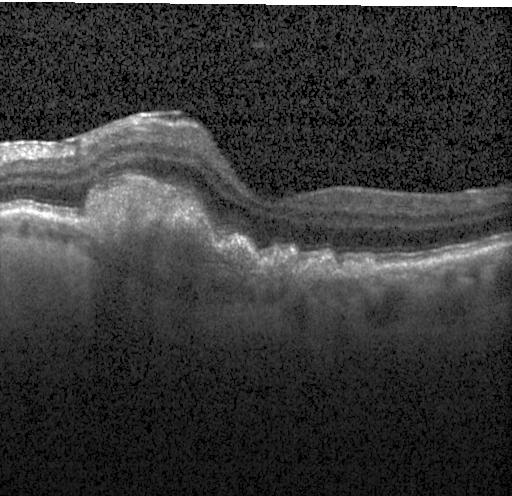 OCT scan showing choroidal neovascularization.